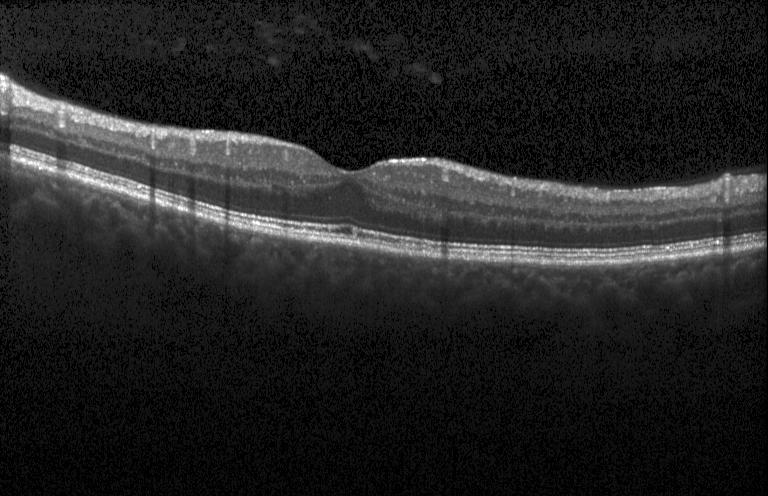

OCT finding: no evidence of choroidal neovascularization, diabetic macular edema, or drusen.